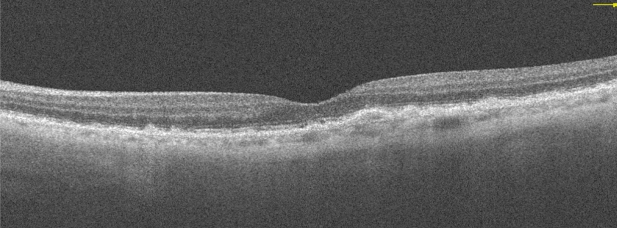
Retinal OCT cross-section. Macular scan.
Impression: age-related macular degeneration (AMD).